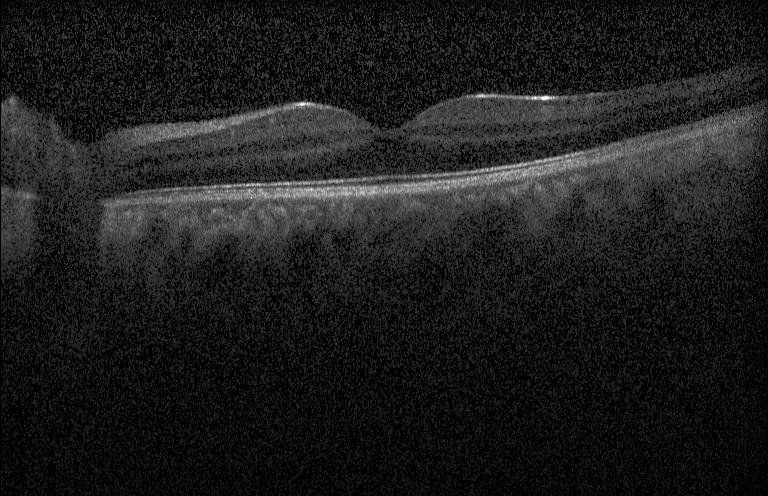 Spectral-domain OCT. Instrument: Heidelberg Spectralis. OCT B-scan
This B-scan demonstrates no CNV, no DME, and no drusen.